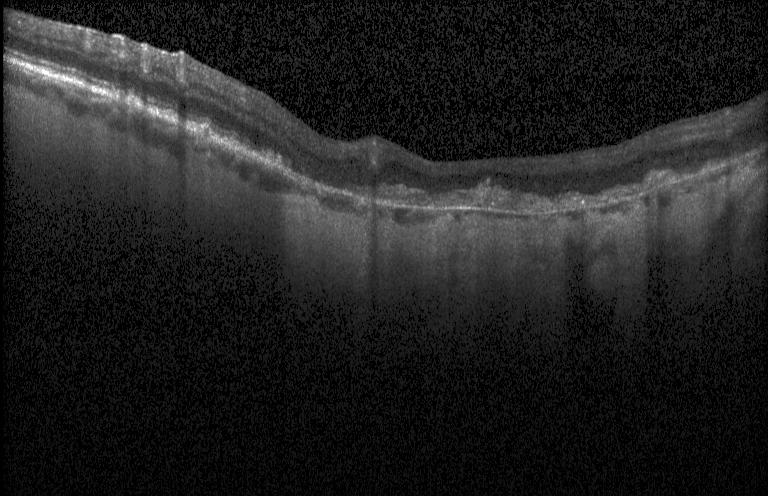 Spectral-domain optical coherence tomography. Optical coherence tomography scan.
Diagnosis: a choroidal neovascular membrane.